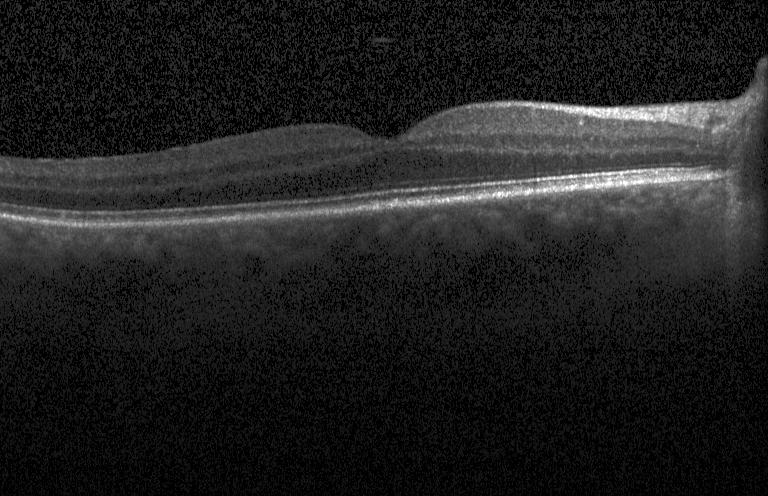
Diagnosis: no CNV, DME, or drusen.